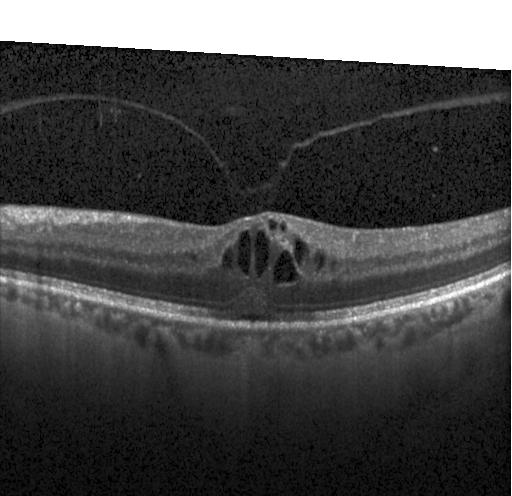

Optical coherence tomography B-scan. Dx: DME.